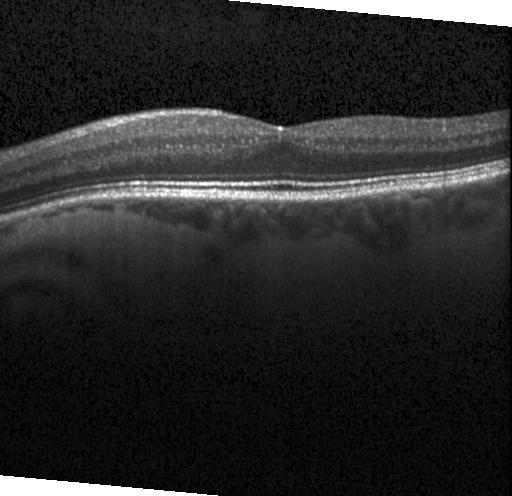 Optical coherence tomography B-scan — Assessment: no choroidal neovascularization, diabetic macular edema, or drusen.